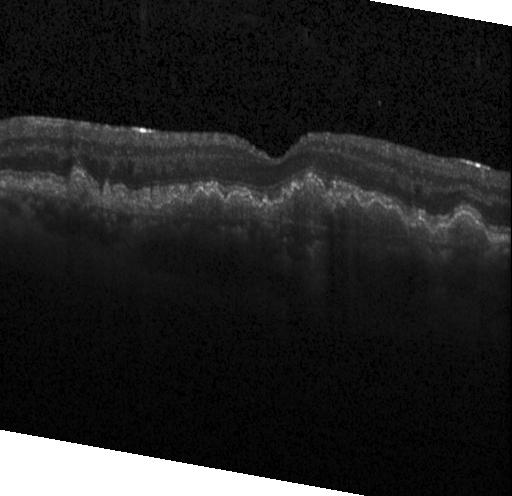 The scan shows a choroidal neovascular membrane.